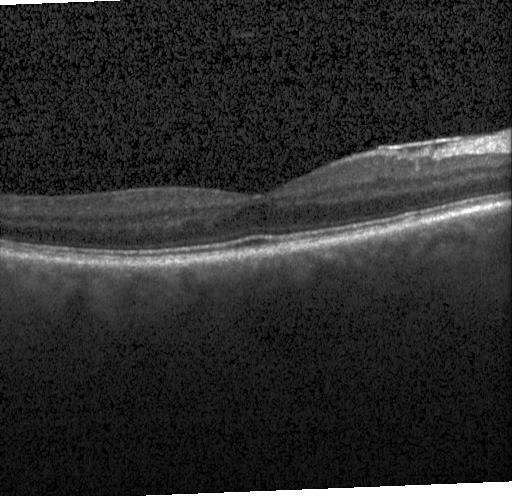 Heidelberg Spectralis OCT system, optical coherence tomography B-scan.
This B-scan demonstrates neither choroidal neovascularization, diabetic macular edema, nor drusen.